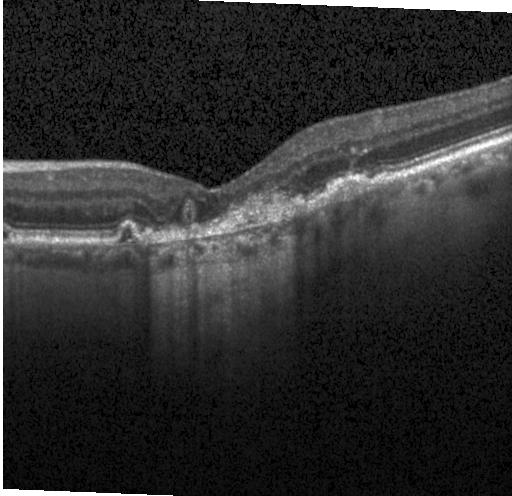

Finding: choroidal neovascularization.